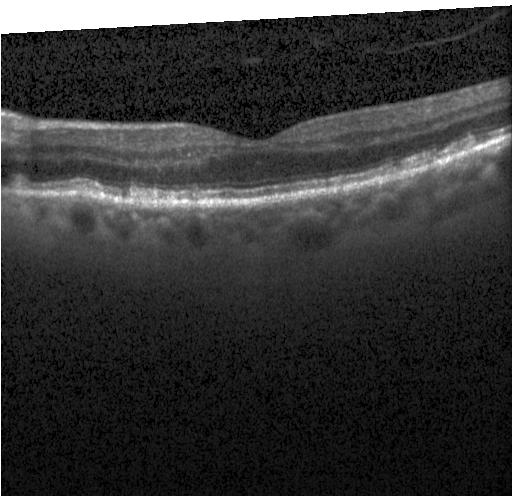
OCT line scan. Impression: sub-RPE drusenoid deposits.